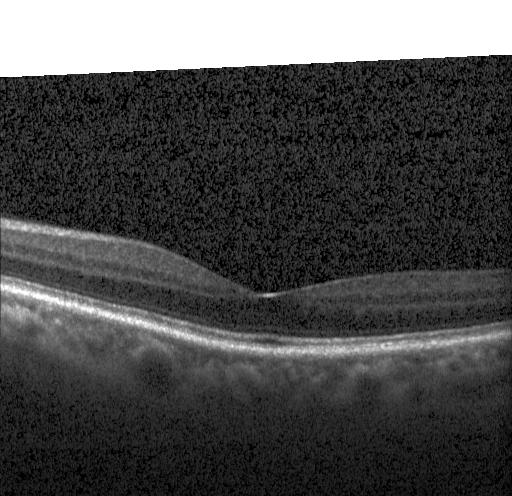
SD-OCT. Fovea-centered. OCT line scan
The scan shows no evidence of choroidal neovascularization, diabetic macular edema, or drusen.